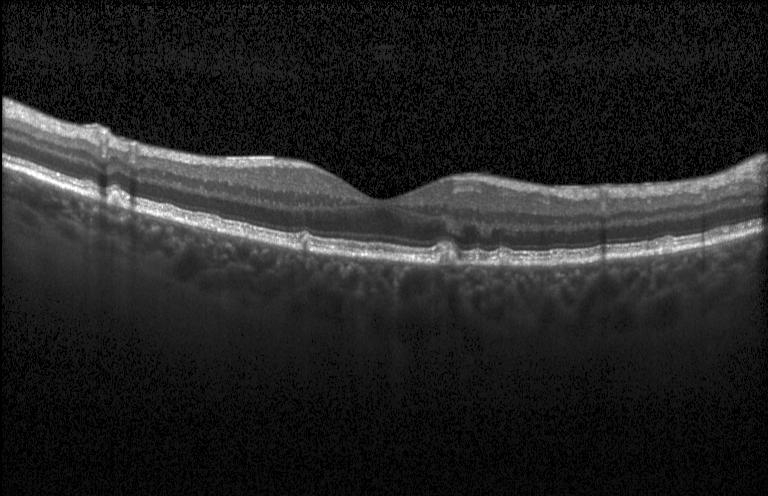

OCT B-scan showing sub-RPE drusenoid deposits.